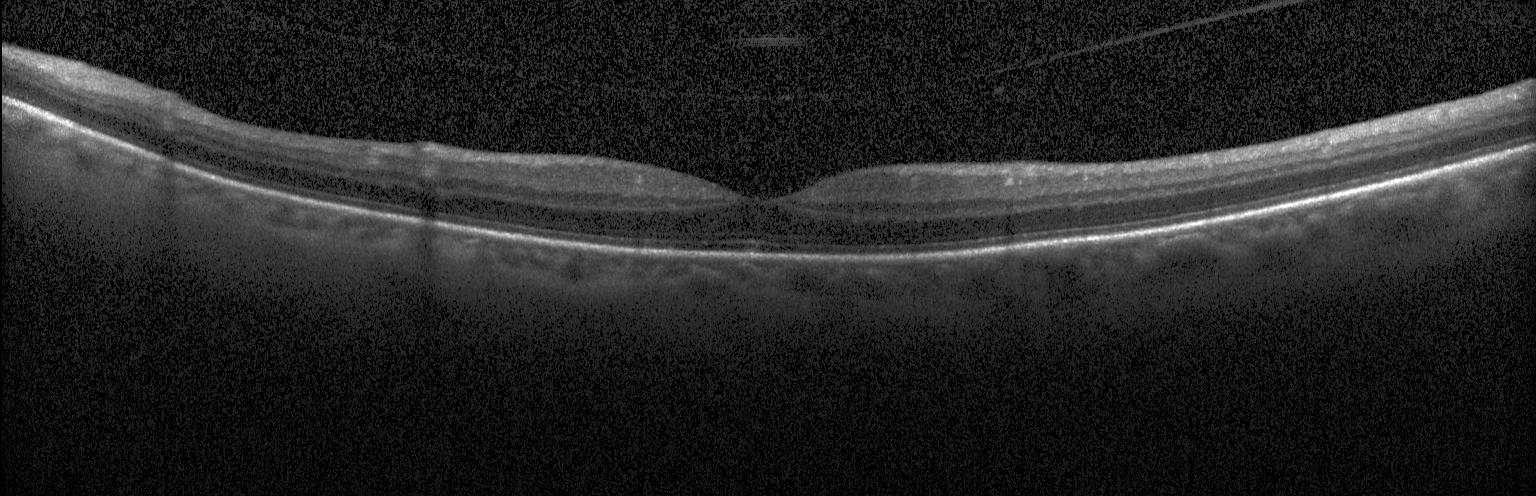

Spectral-domain OCT B-scan: neither choroidal neovascularization, diabetic macular edema, nor drusen.